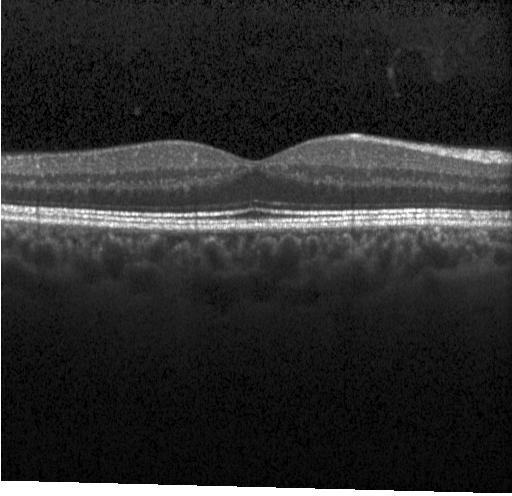

Optical coherence tomography B-scan. Diagnosis: no evidence of choroidal neovascularization, diabetic macular edema, or drusen.